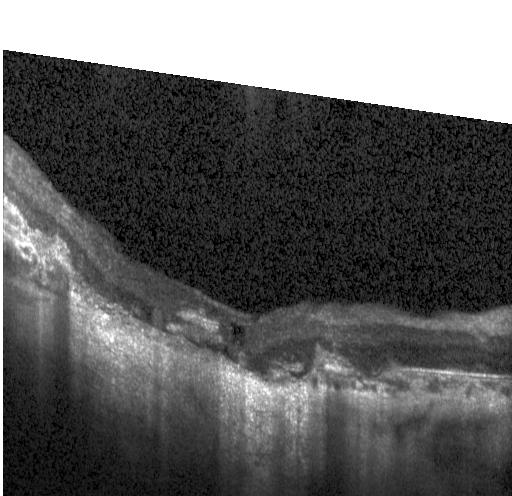
A choroidal neovascular membrane.